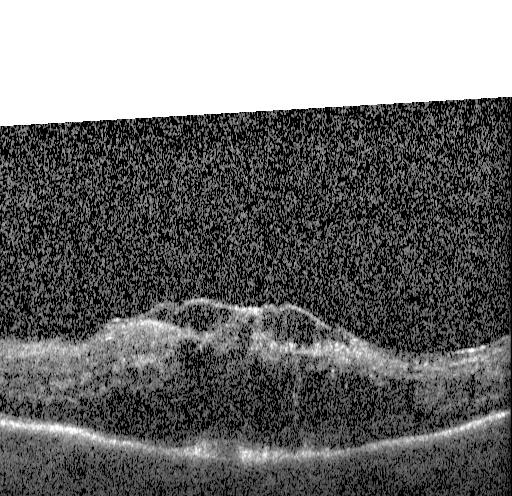
Finding: diabetic macular edema.